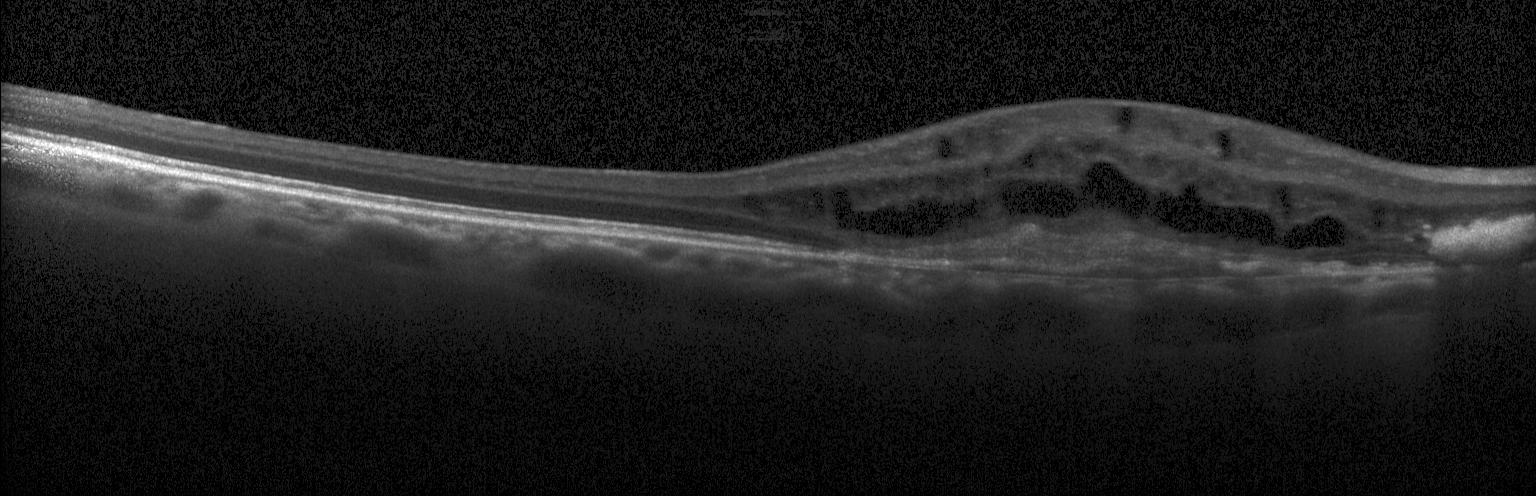
Retinal OCT cross-section showing a choroidal neovascular membrane.